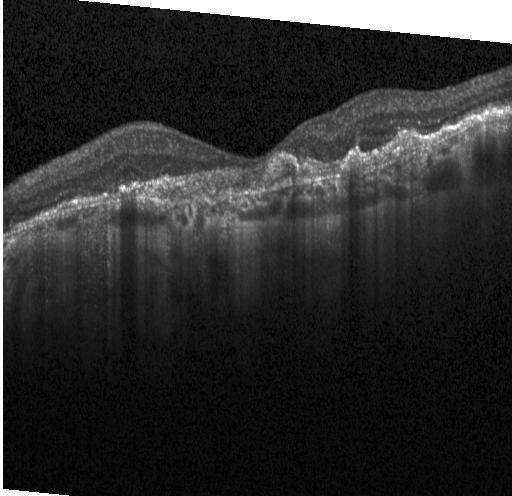 Retinal OCT cross-section, macular scan, spectral-domain optical coherence tomography — Diagnosis: a choroidal neovascular membrane.